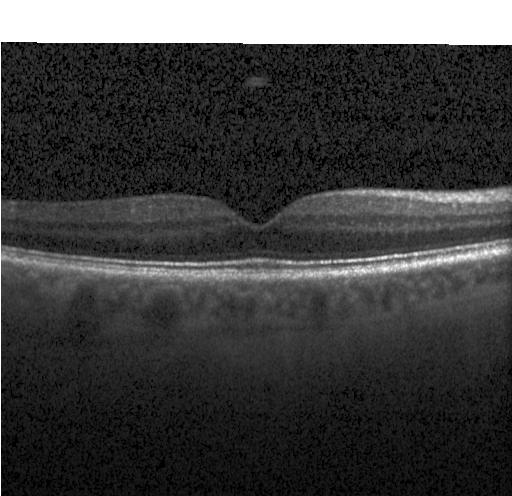 Finding: no evidence of choroidal neovascularization, diabetic macular edema, or drusen.